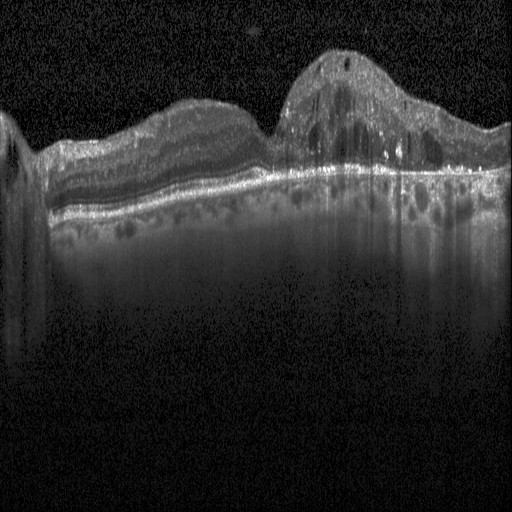

Spectral-domain optical coherence tomography. Optical coherence tomography B-scan. Fovea-centered. DME.